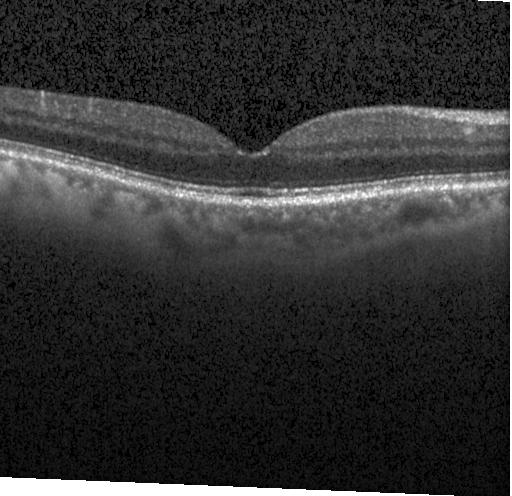
Spectral-domain OCT B-scan: no choroidal neovascularization, diabetic macular edema, or drusen.